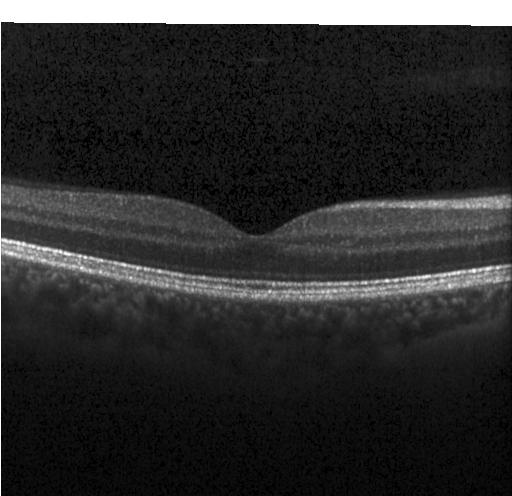 Macular scan; retinal OCT cross-section. Dx: no choroidal neovascularization, no diabetic macular edema, and no drusen.